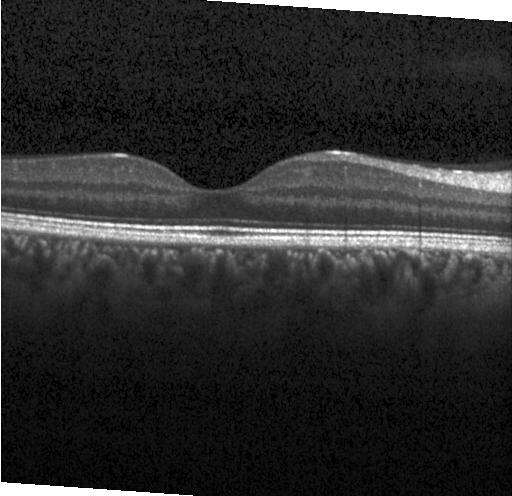 Impression: no CNV, DME, or drusen.